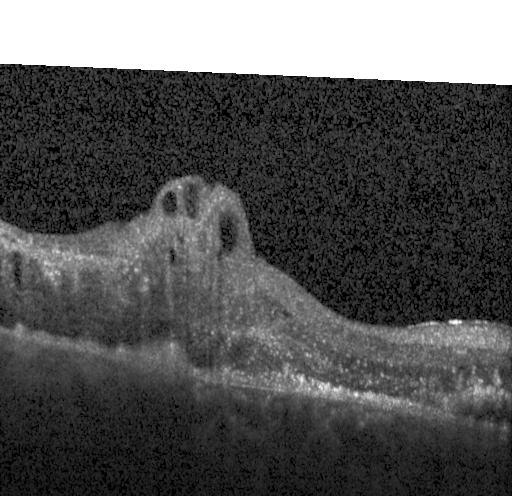

Impression: a choroidal neovascular membrane.